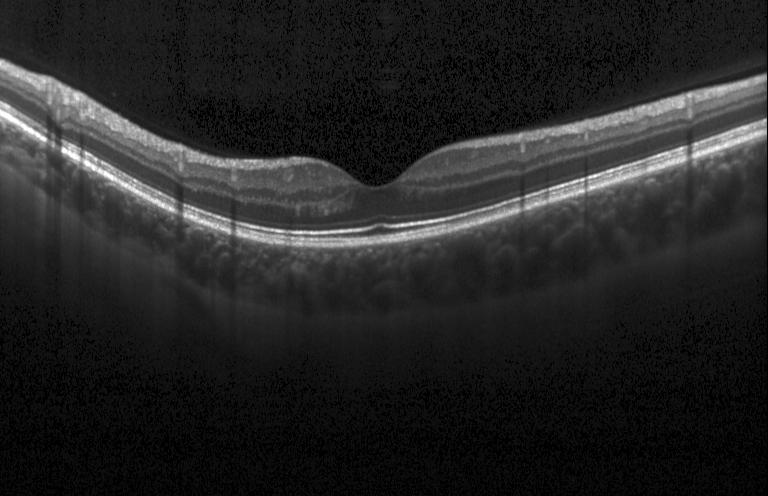 Macular OCT: no choroidal neovascularization, diabetic macular edema, or drusen.